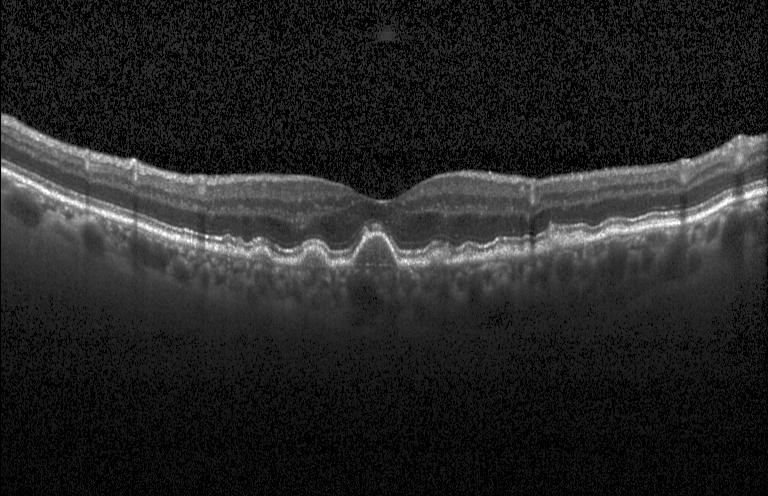 OCT B-scan.
Finding: multiple drusen.